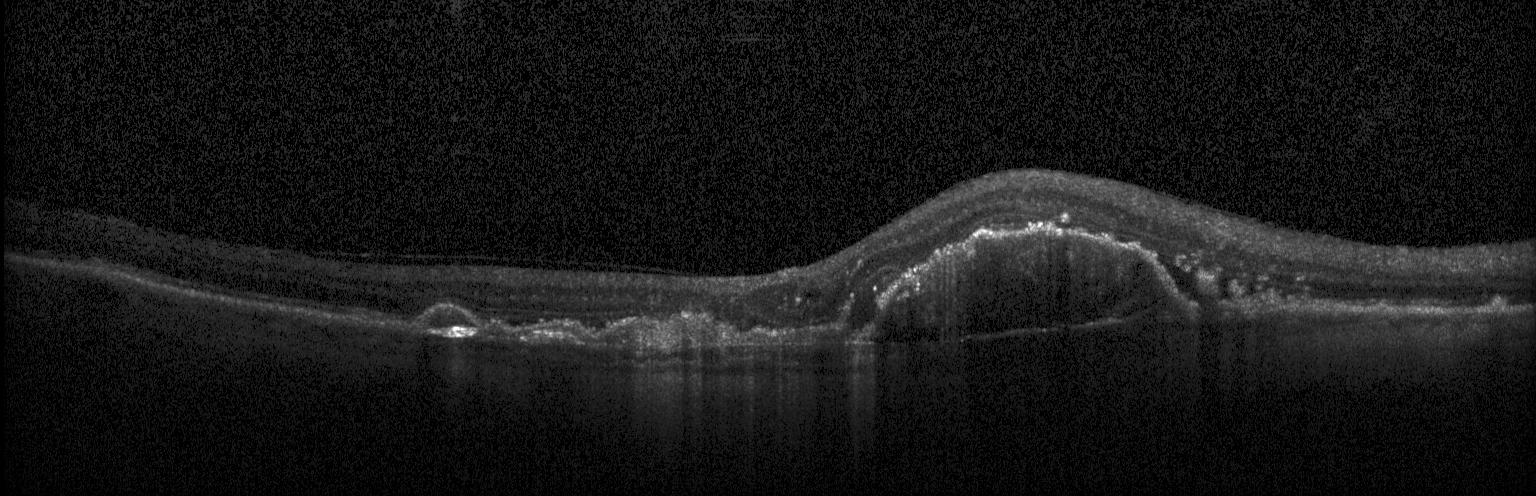
Horizontal scan through the fovea. Retinal OCT B-scan. Spectral-domain OCT. Instrument: Heidelberg Spectralis
Diagnosis: a choroidal neovascular membrane.